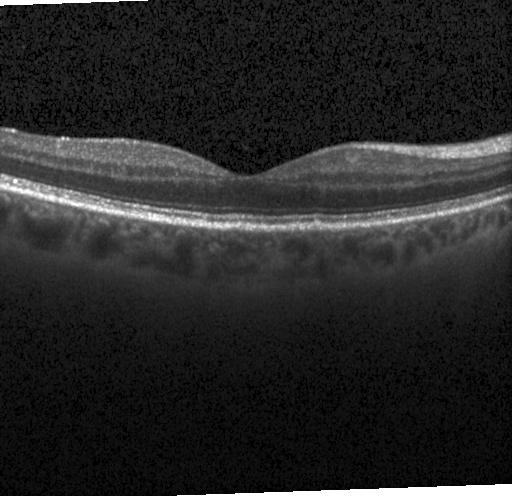
Optical coherence tomography B-scan — Finding: no evidence of choroidal neovascularization, diabetic macular edema, or drusen.